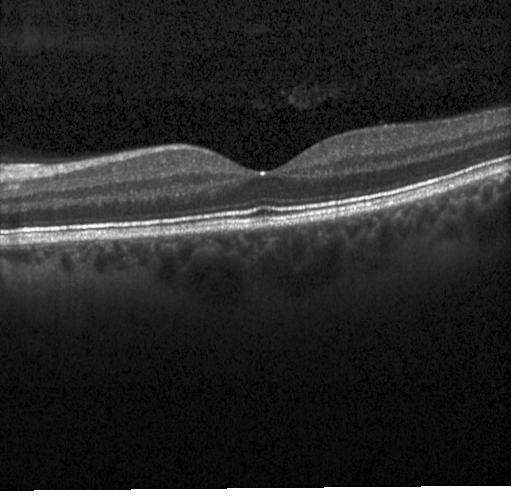

Centered on the fovea; optical coherence tomography scan; acquired on a Heidelberg Spectralis; SD-OCT
Finding: no choroidal neovascularization, no diabetic macular edema, and no drusen.